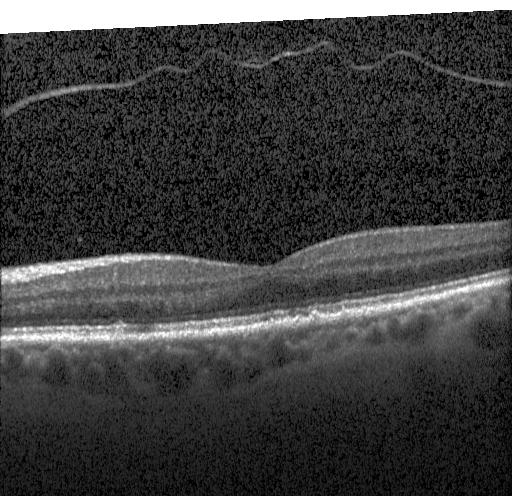 Acquired on a Heidelberg Spectralis, spectral-domain optical coherence tomography, macular scan, optical coherence tomography B-scan.
This B-scan demonstrates drusen.